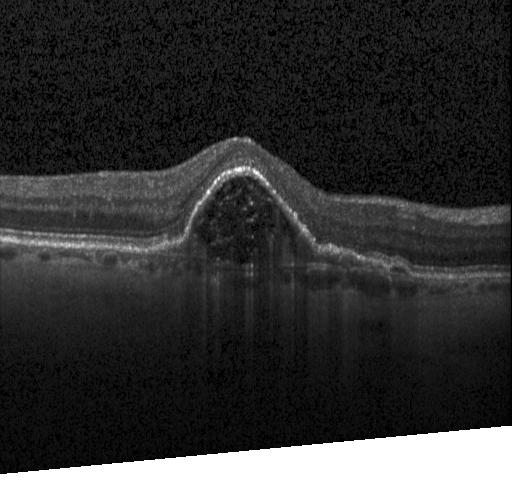 Dx: a choroidal neovascular membrane.